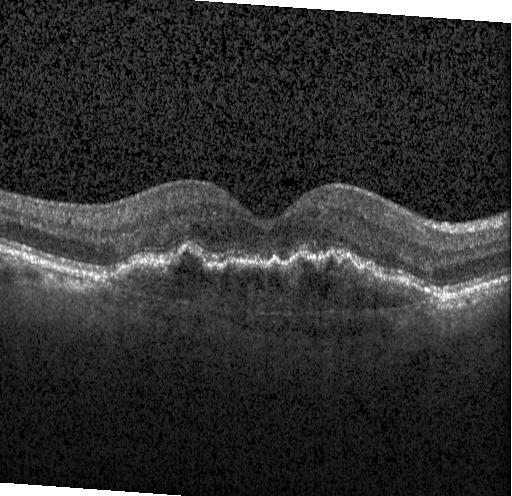

OCT B-scan, spectral-domain optical coherence tomography
Finding: choroidal neovascularization.